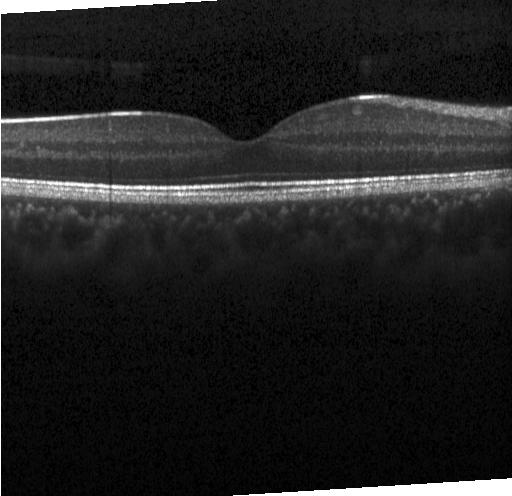

Spectral-domain OCT B-scan: no CNV, no DME, and no drusen.